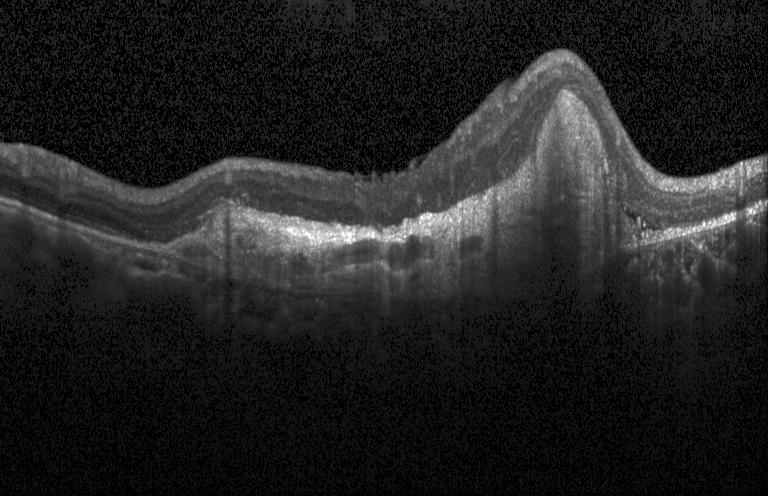

Finding: choroidal neovascularization.